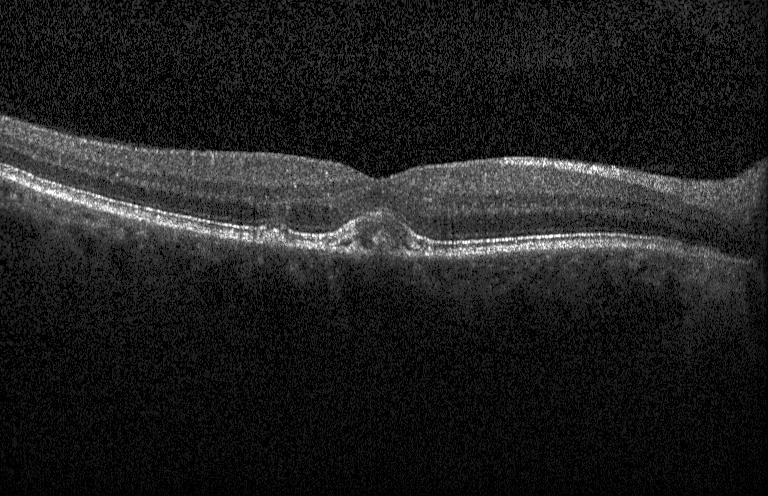
Finding: CNV.